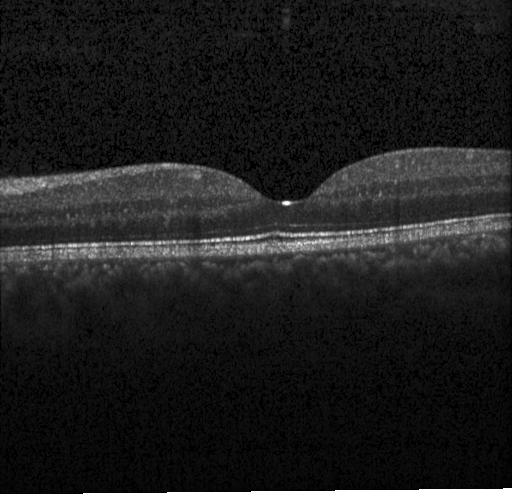 Macular OCT: no choroidal neovascularization, diabetic macular edema, or drusen.